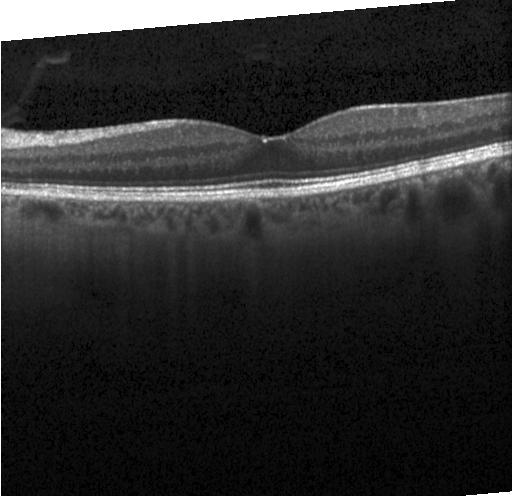
Impression: no evidence of CNV, DME, or drusen.